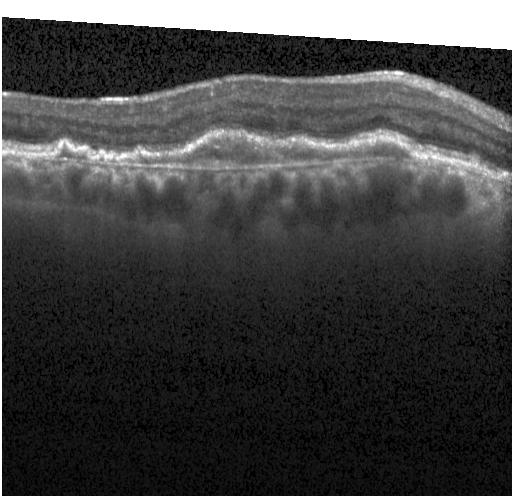
Spectral-domain optical coherence tomography, OCT B-scan, centered on the fovea
Finding: choroidal neovascularization.